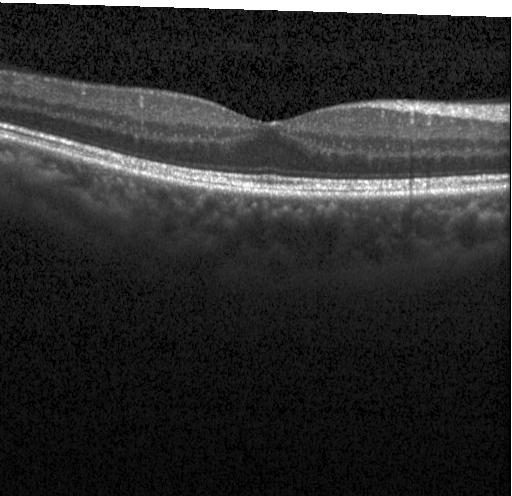

Instrument: Heidelberg Spectralis; horizontal scan through the fovea; SD-OCT; retinal OCT cross-section.
No choroidal neovascularization, no diabetic macular edema, and no drusen.